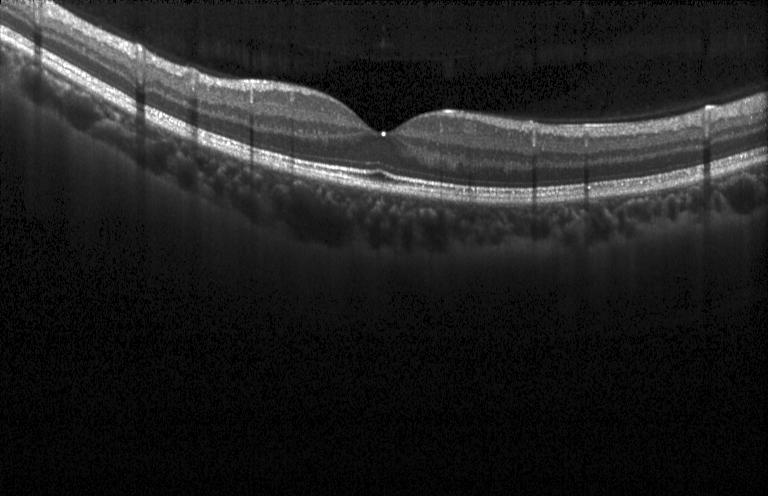
No choroidal neovascularization, diabetic macular edema, or drusen.